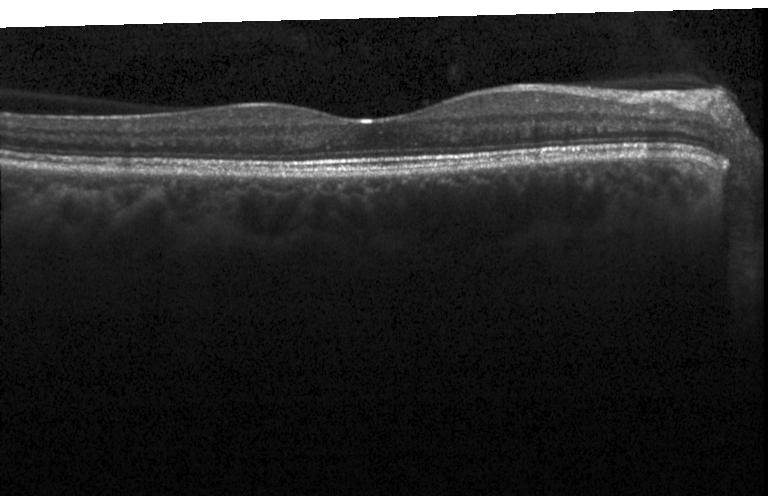

SD-OCT, through the macula, acquired on a Heidelberg Spectralis, retinal OCT B-scan.
This B-scan demonstrates no choroidal neovascularization, no diabetic macular edema, and no drusen.